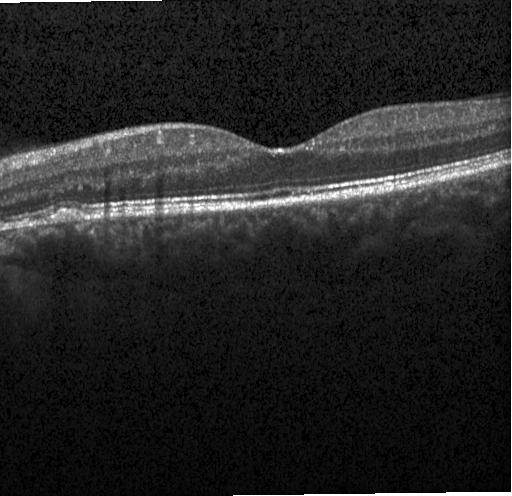

Optical coherence tomography B-scan
Diagnosis: drusen.